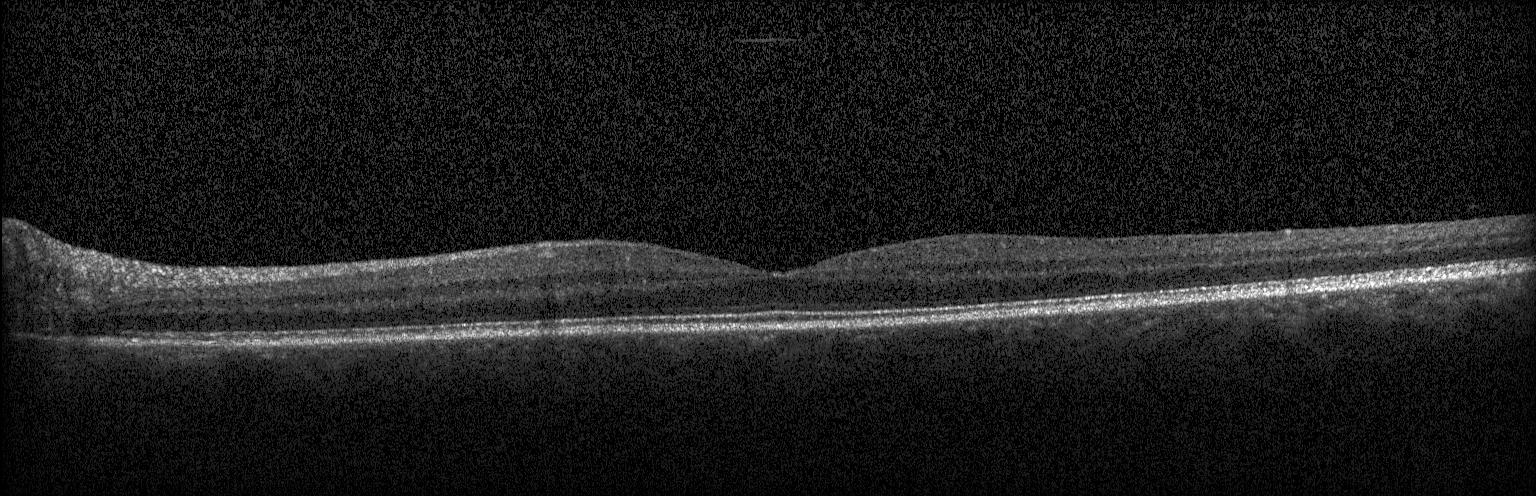 Diagnosis: no evidence of choroidal neovascularization, diabetic macular edema, or drusen.